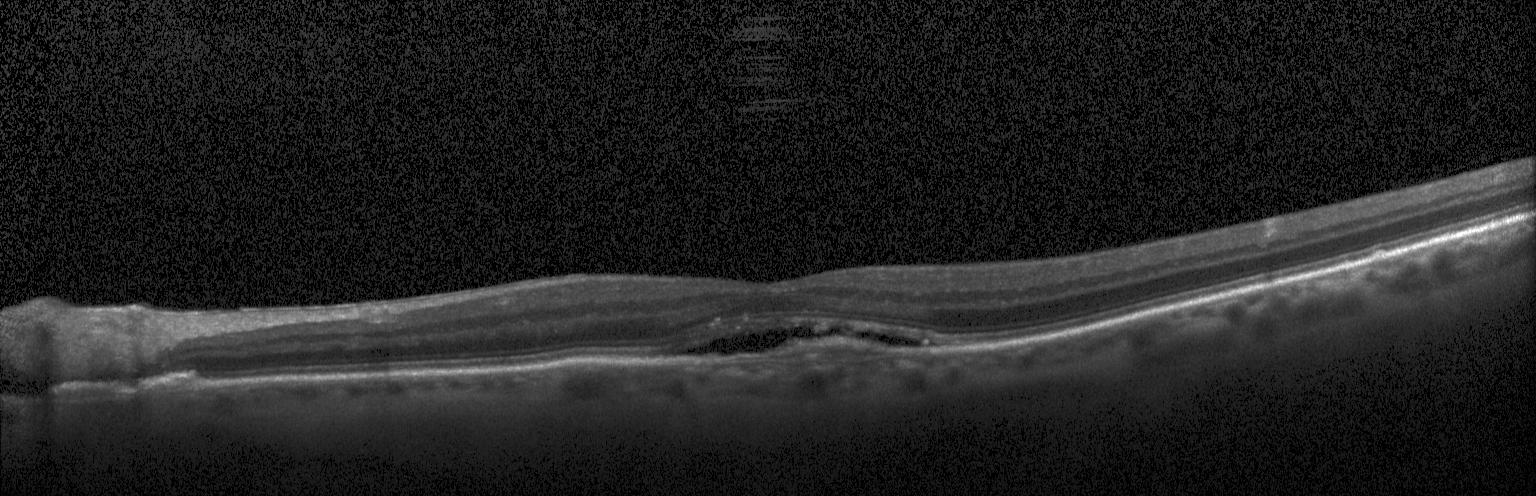 Dx: choroidal neovascularization.